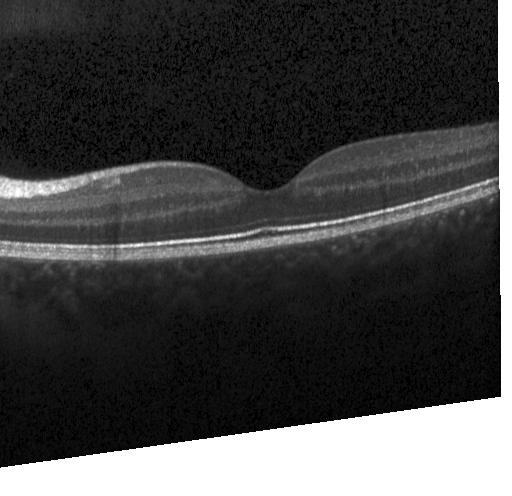

OCT line scan — Finding: no choroidal neovascularization, no diabetic macular edema, and no drusen.